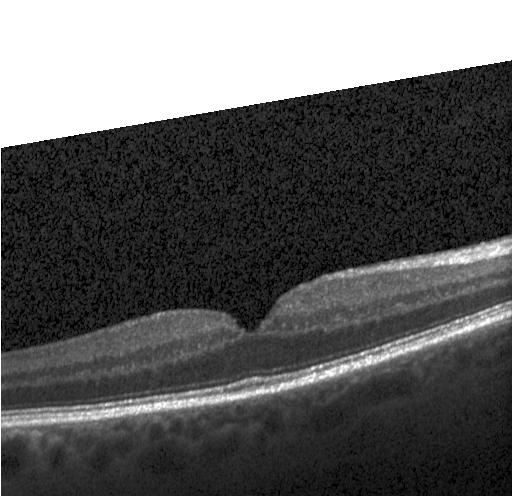 Spectral-domain optical coherence tomography · Heidelberg Spectralis · horizontal scan through the fovea · OCT B-scan
Assessment: neither choroidal neovascularization, diabetic macular edema, nor drusen.